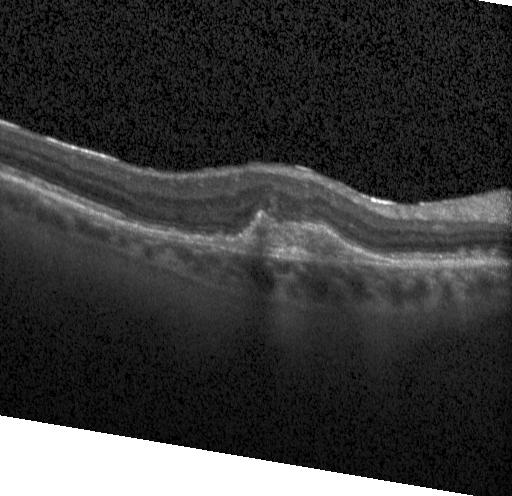
Spectral-domain optical coherence tomography. Retinal OCT B-scan. Horizontal scan through the fovea. Acquired on a Heidelberg Spectralis.
Diagnosis: choroidal neovascularization (CNV).